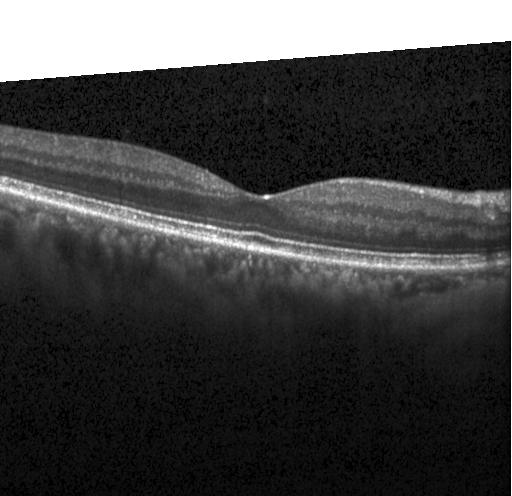
Finding: no choroidal neovascularization, diabetic macular edema, or drusen.